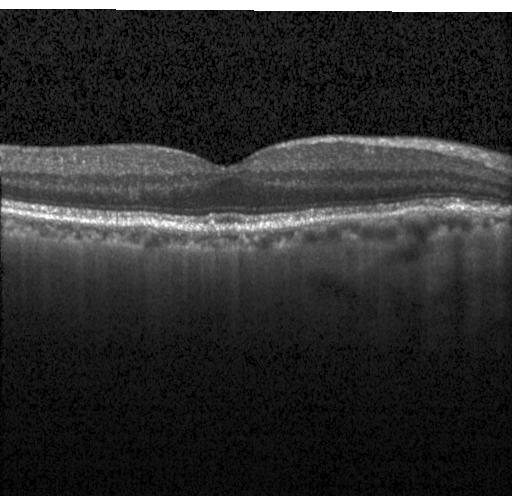 The scan shows sub-RPE drusenoid deposits.